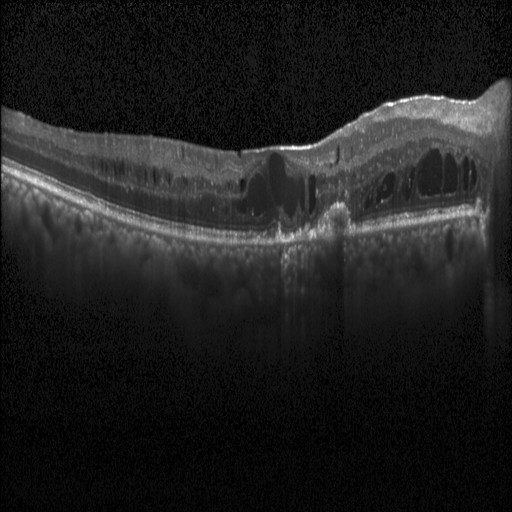
Retinal OCT cross-section showing diabetic macular edema (DME).